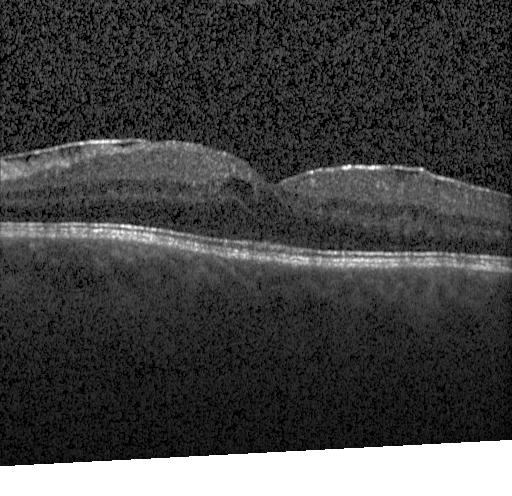
Acquired on a Heidelberg Spectralis; fovea-centered; OCT line scan
Impression: diabetic macular edema (DME).